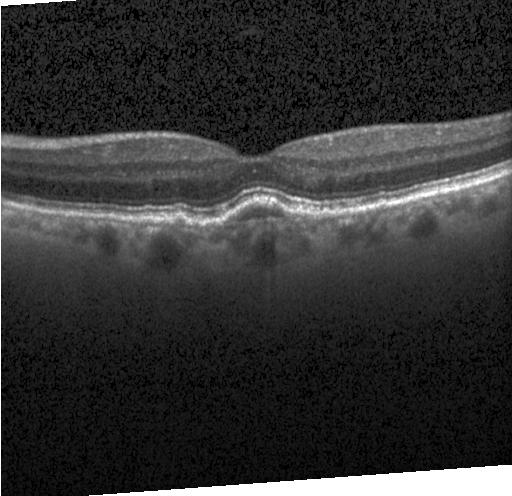
Finding: a choroidal neovascular membrane.